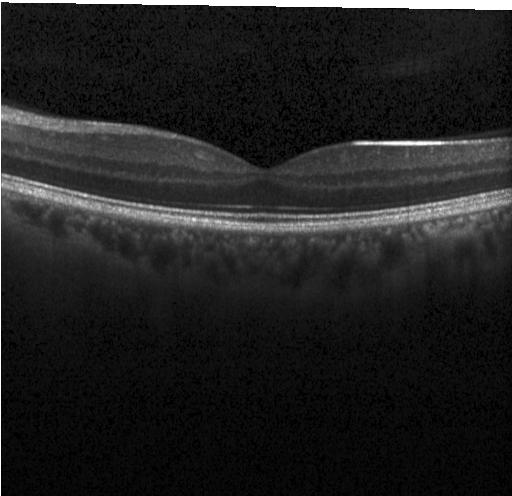
No choroidal neovascularization, diabetic macular edema, or drusen.